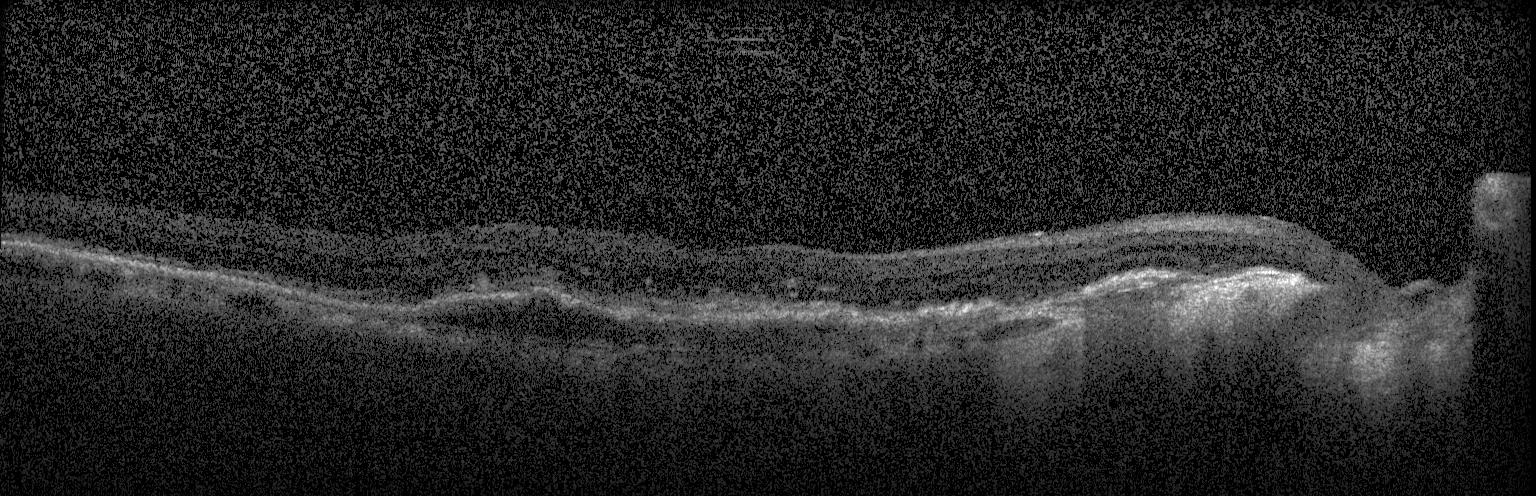
This B-scan demonstrates a choroidal neovascular membrane.